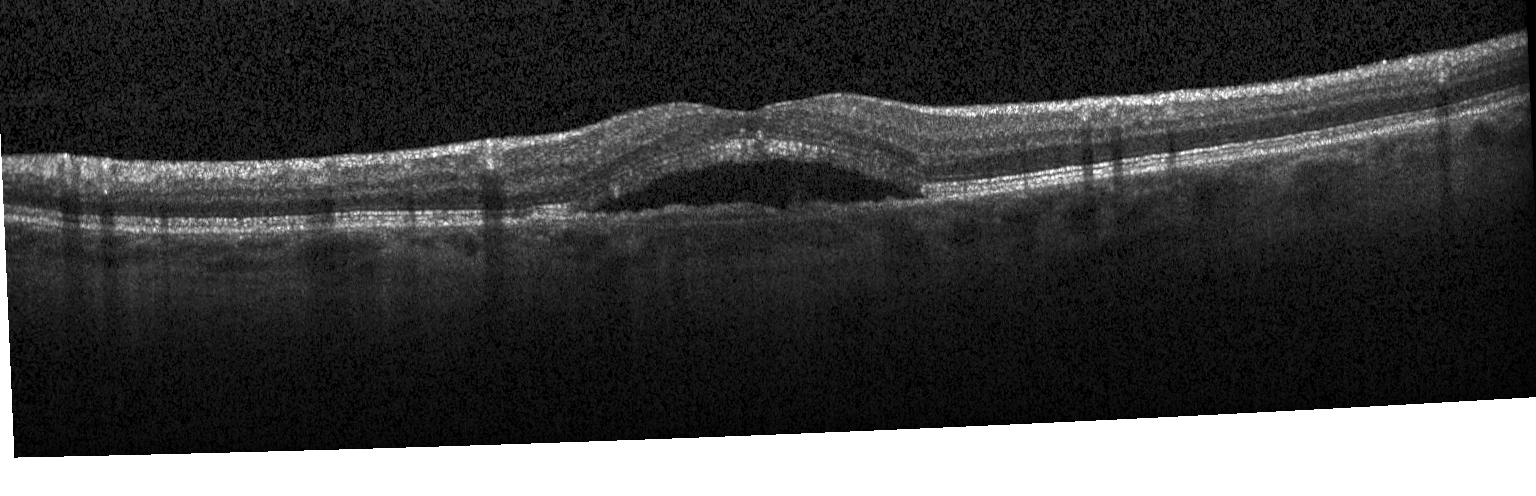 Dx: choroidal neovascularization.